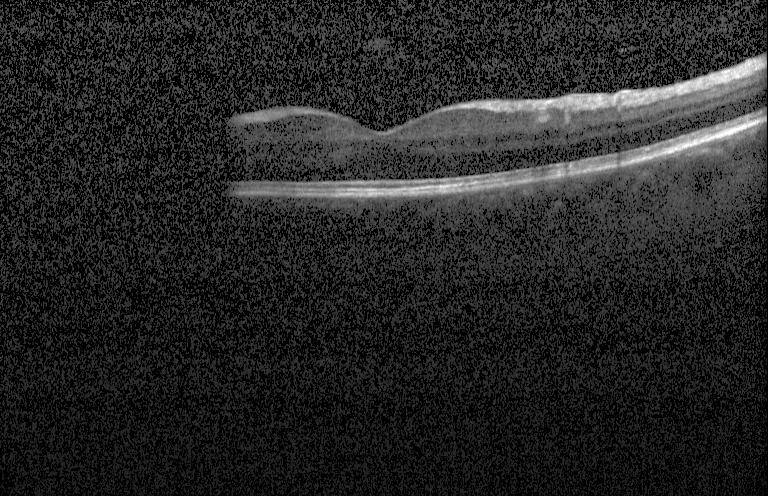
Impression: neither CNV, DME, nor drusen.